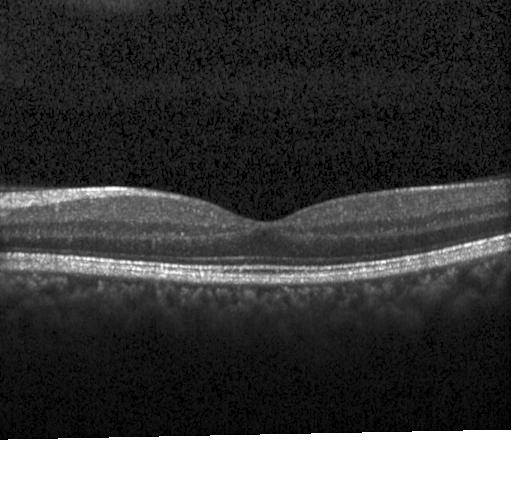 Diagnosis: no evidence of CNV, DME, or drusen.